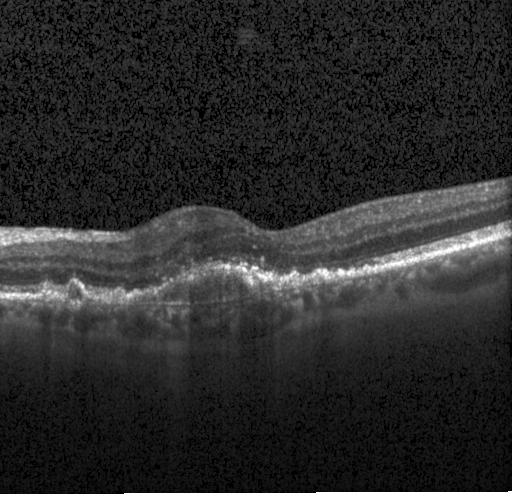

Retinal OCT cross-section
Diagnosis: choroidal neovascularization (CNV).